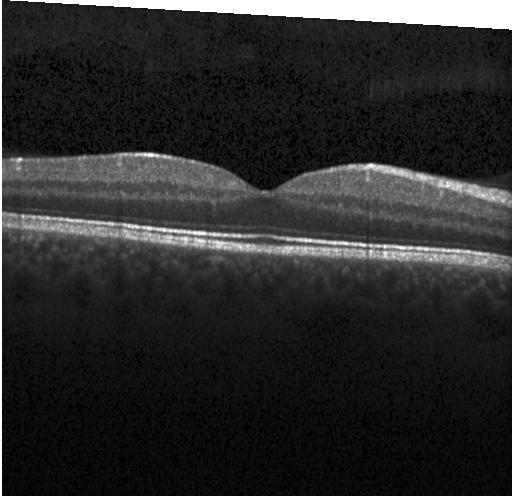
Optical coherence tomography B-scan. Centered on the fovea.
Diagnosis: no choroidal neovascularization, diabetic macular edema, or drusen.